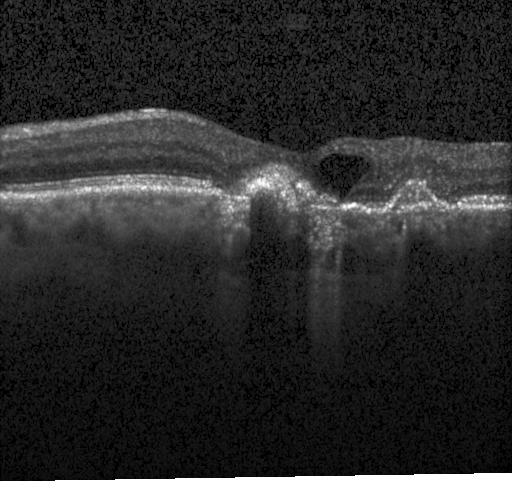 Horizontal scan through the fovea. OCT line scan. Spectral-domain optical coherence tomography.
This B-scan demonstrates a choroidal neovascular membrane.